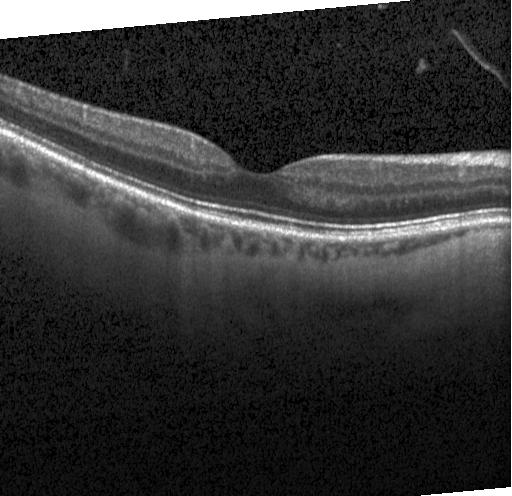
Retinal OCT cross-section
No evidence of CNV, DME, or drusen.